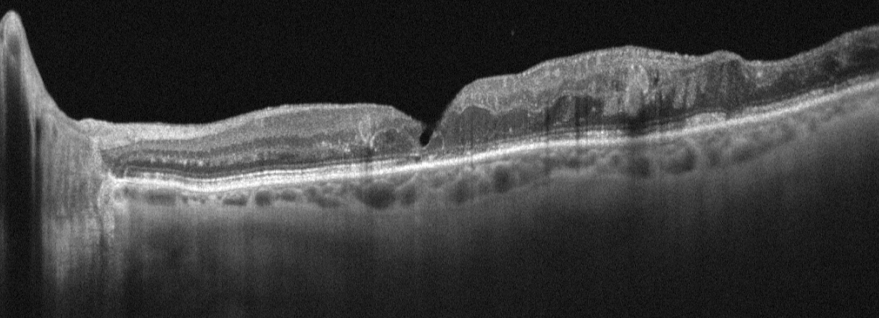
Optical coherence tomography scan · macular scan · acquired on an Optovue Avanti RTVue XR. Dx: diabetic macular edema (DME).